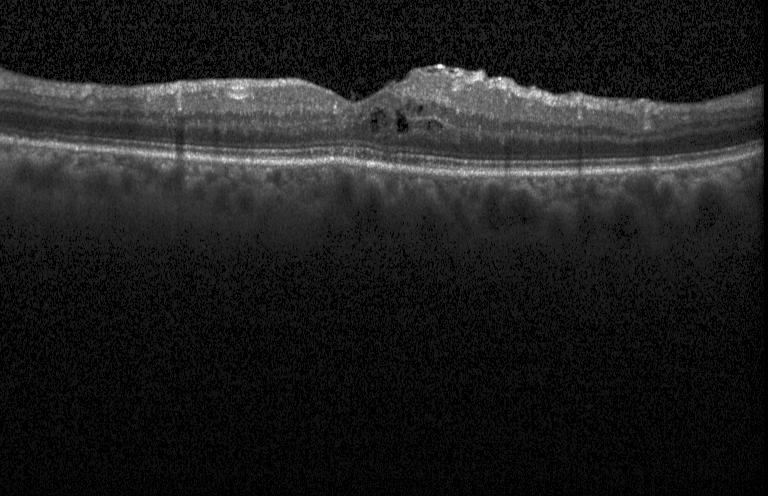
Finding: diabetic macular edema (DME).